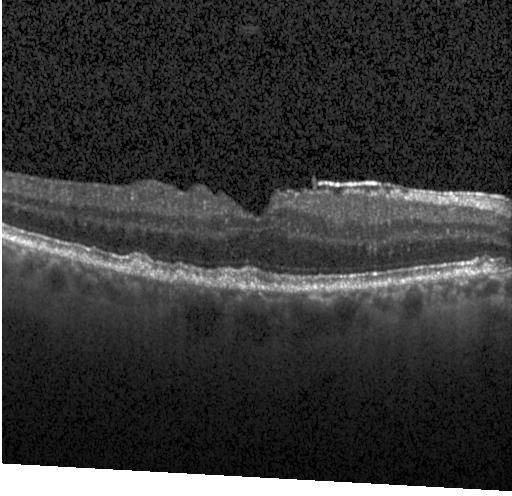 Optical coherence tomography scan. Acquired on a Heidelberg Spectralis. Spectral-domain optical coherence tomography.
Impression: multiple drusen.